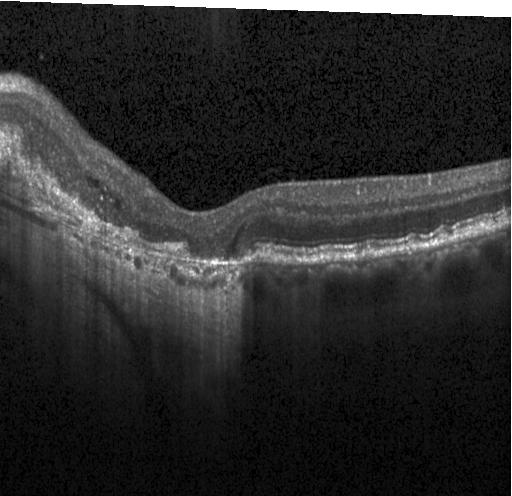 Dx: choroidal neovascularization.